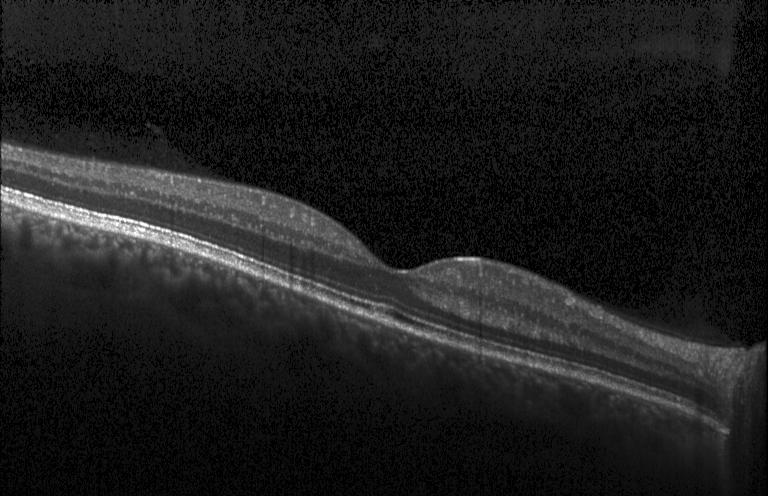
Through the macula. Retinal OCT B-scan.
Macular OCT: no CNV, no DME, and no drusen.